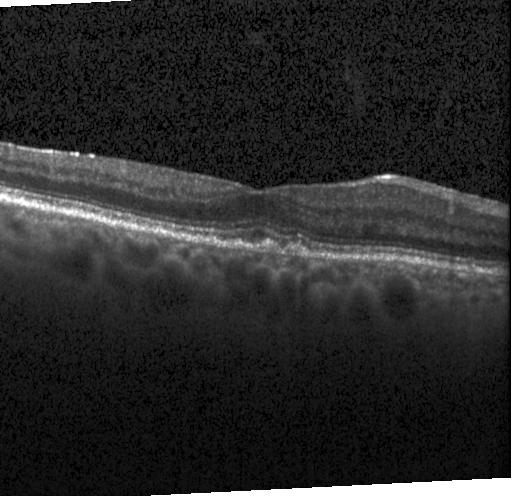

Spectral-domain OCT · optical coherence tomography B-scan.
The scan shows drusen.